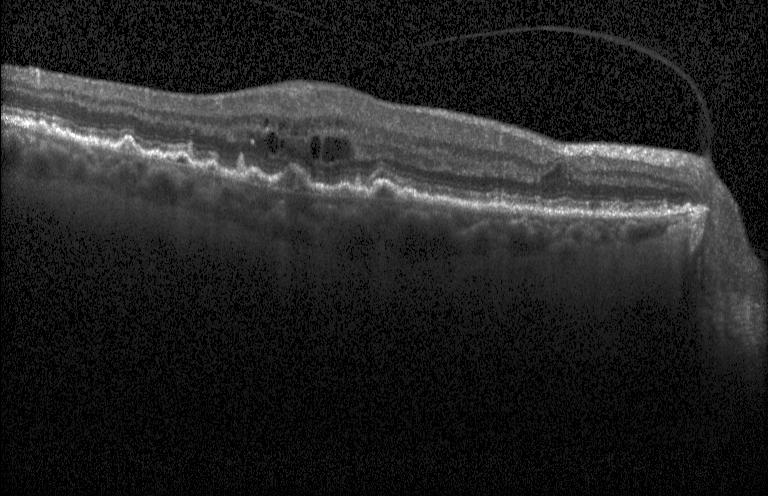 Optical coherence tomography B-scan. Spectral-domain optical coherence tomography. Fovea-centered. A choroidal neovascular membrane.